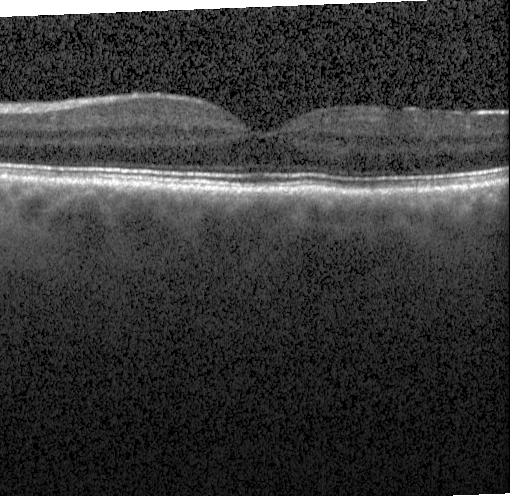
Acquired on a Heidelberg Spectralis. Retinal OCT B-scan. Centered on the fovea. Spectral-domain optical coherence tomography
Diagnosis: no evidence of CNV, DME, or drusen.